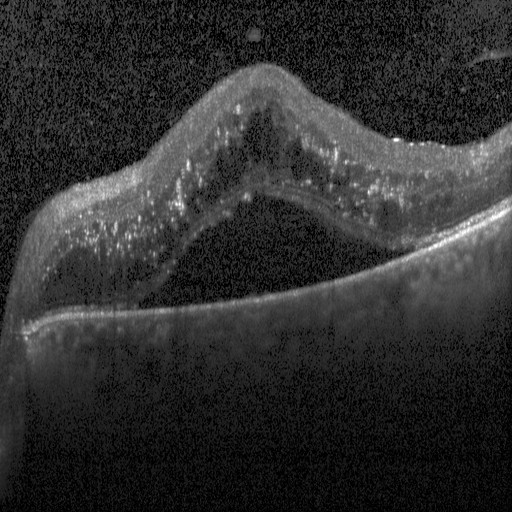

OCT B-scan. Dx: DME.